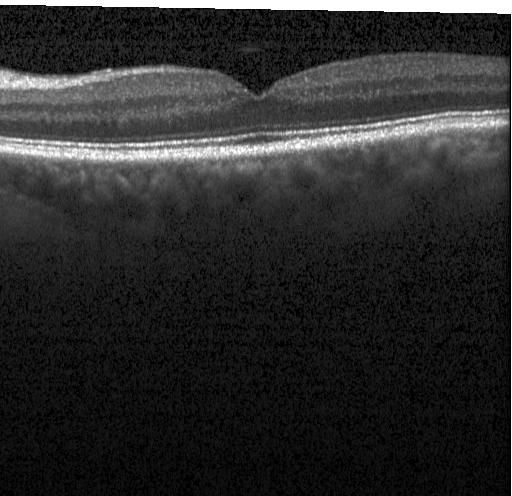
OCT line scan
Impression: no choroidal neovascularization, diabetic macular edema, or drusen.